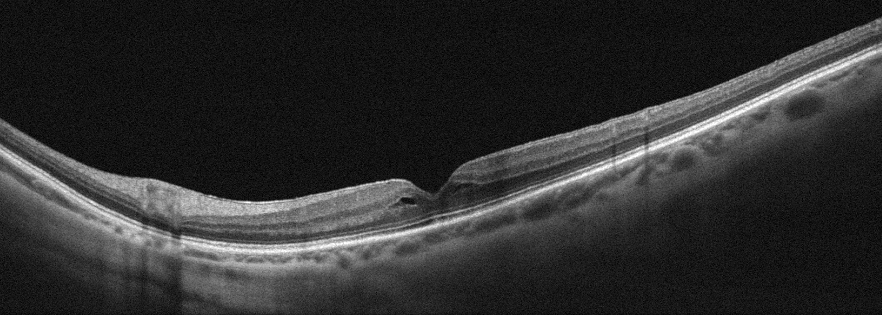 OCT B-scan, oculus sinister — Vitreomacular interface disease.